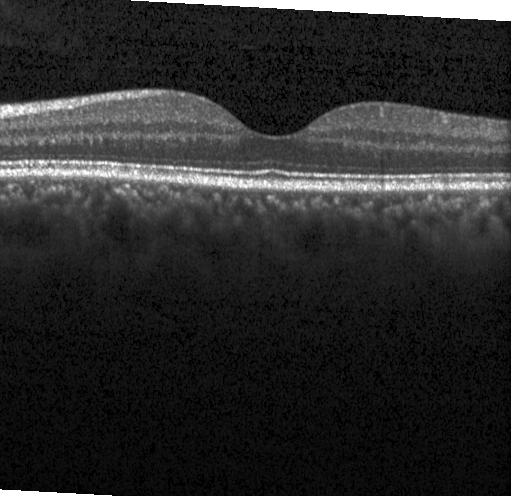
Retinal OCT B-scan. Finding: no choroidal neovascularization, diabetic macular edema, or drusen.